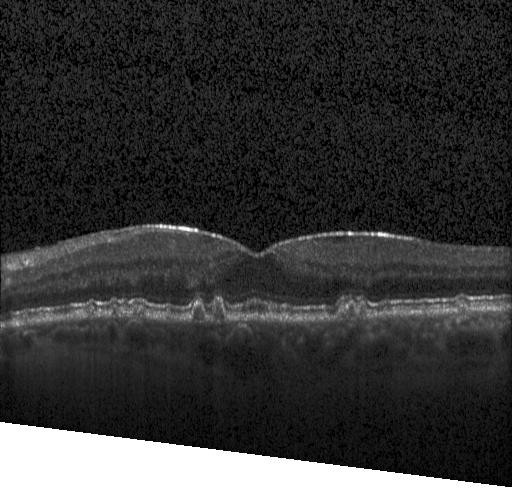 Dx: drusen.